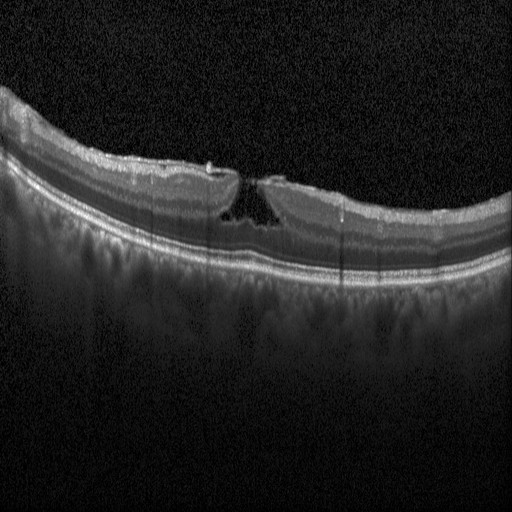 Assessment: DME.